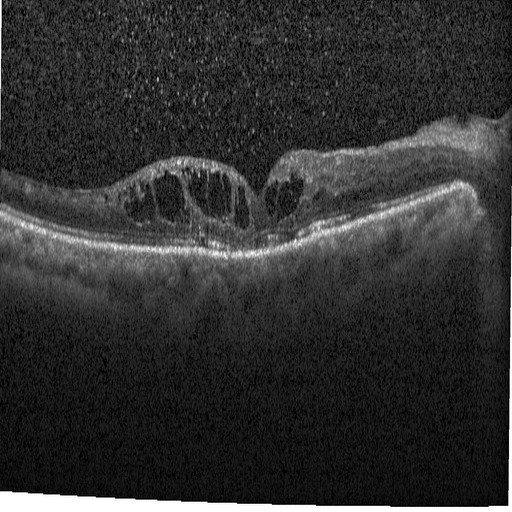 SD-OCT, retinal OCT cross-section, Heidelberg Spectralis, macular scan. Finding: diabetic macular edema (DME).